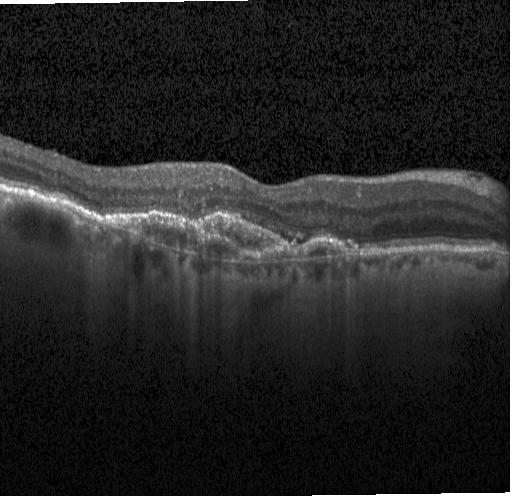 Optical coherence tomography B-scan — This B-scan demonstrates a choroidal neovascular membrane.